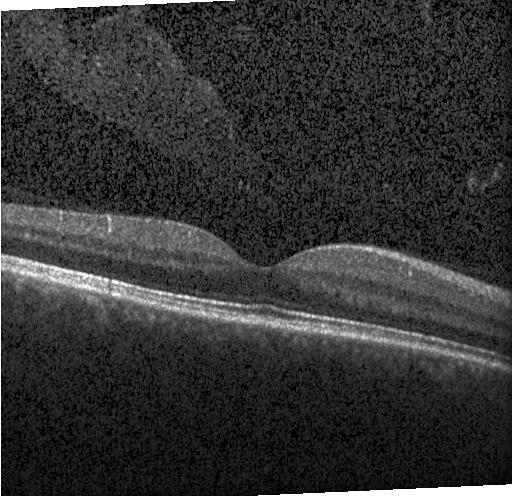

Impression: no evidence of choroidal neovascularization, diabetic macular edema, or drusen.